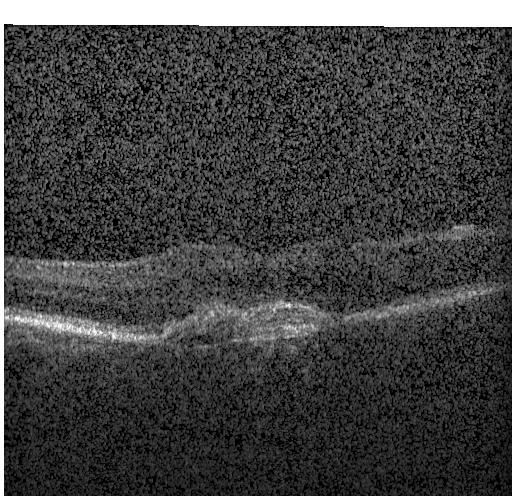 Fovea-centered, OCT line scan, acquired on a Heidelberg Spectralis
Impression: choroidal neovascularization.